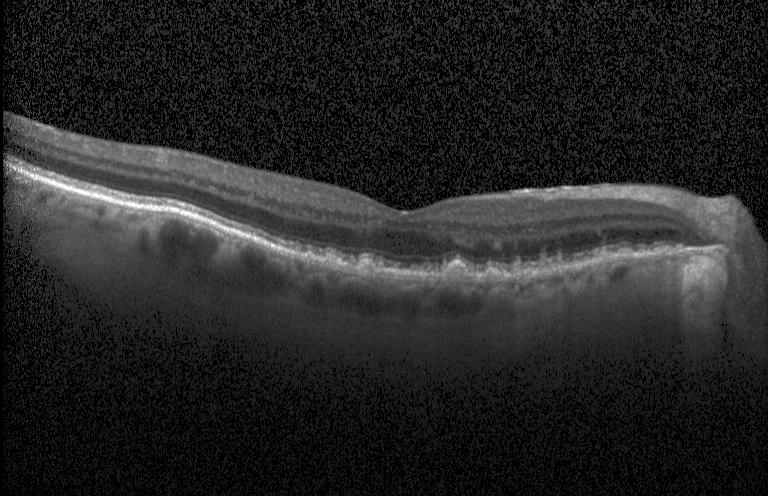
Heidelberg Spectralis OCT system, optical coherence tomography scan, SD-OCT — Assessment: sub-RPE drusenoid deposits.